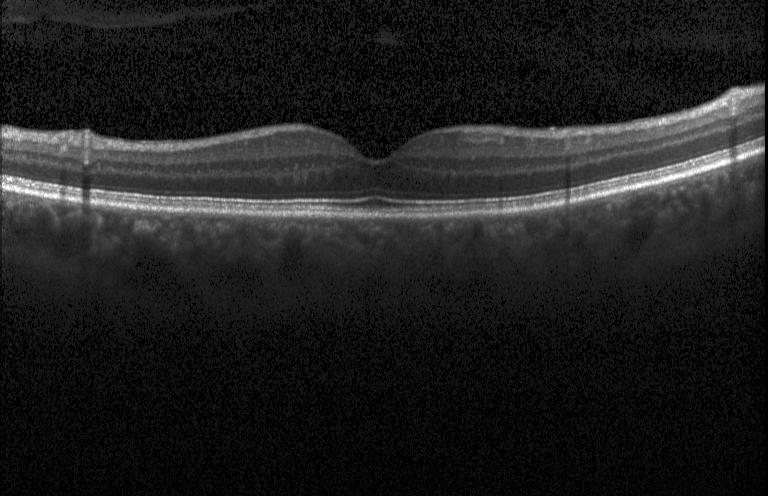 No CNV, no DME, and no drusen.